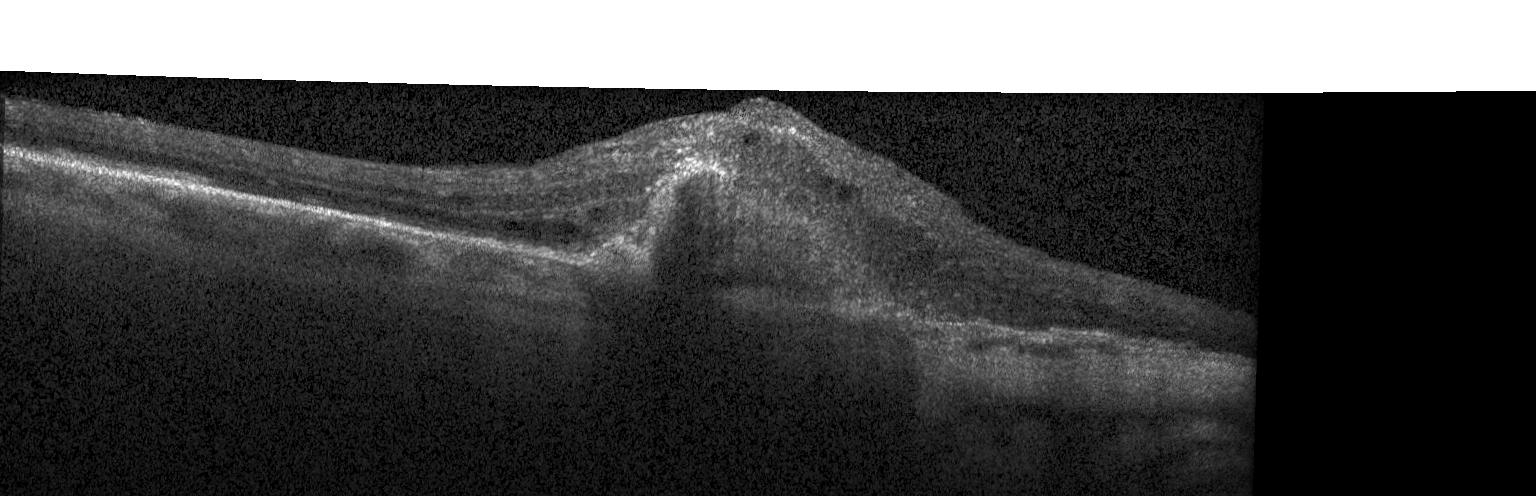
Optical coherence tomography B-scan, Heidelberg Spectralis
A choroidal neovascular membrane.